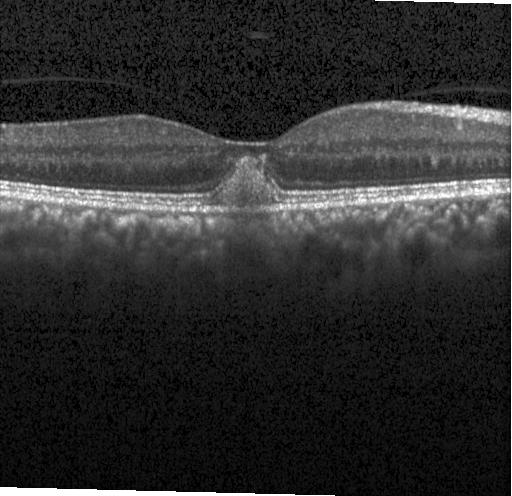
Spectral-domain OCT, retinal OCT cross-section
The scan shows a choroidal neovascular membrane.